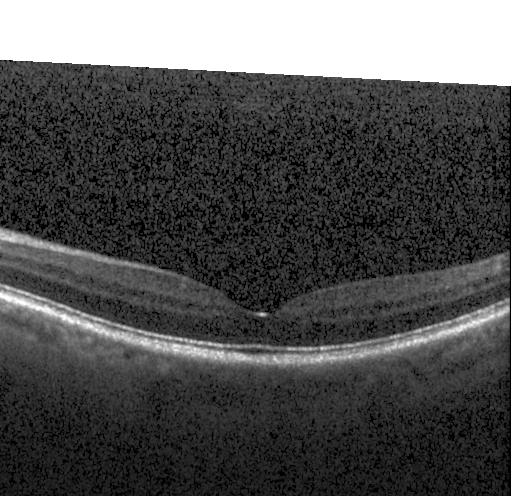 Optical coherence tomography B-scan · Heidelberg Spectralis.
Assessment: no evidence of choroidal neovascularization, diabetic macular edema, or drusen.